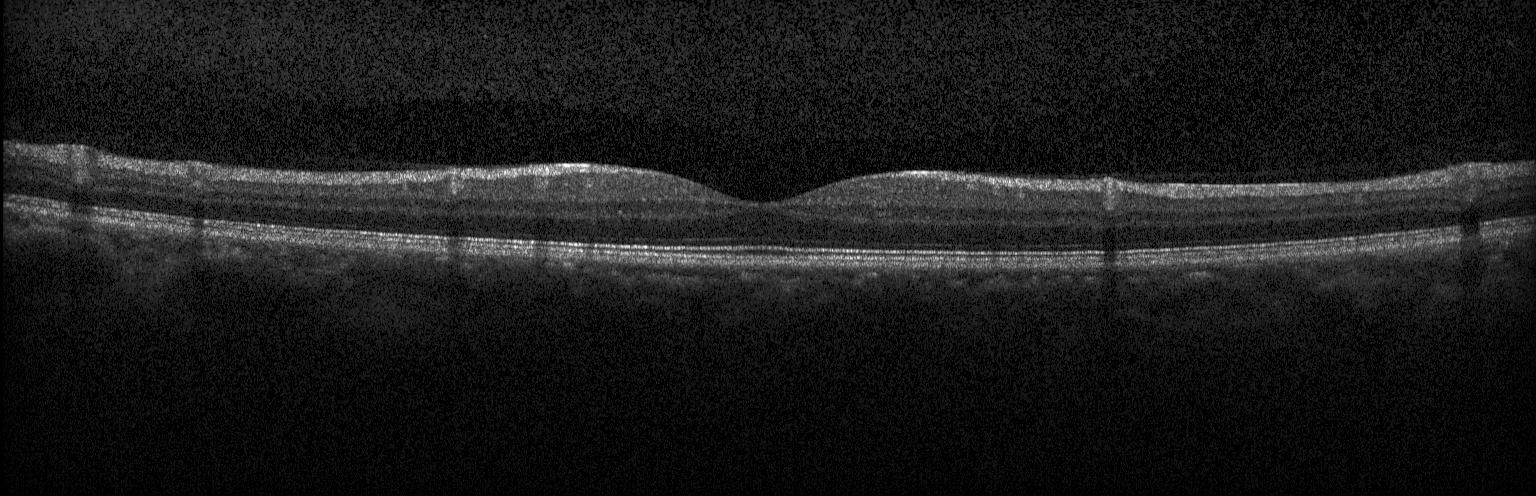
The scan shows no choroidal neovascularization, diabetic macular edema, or drusen.